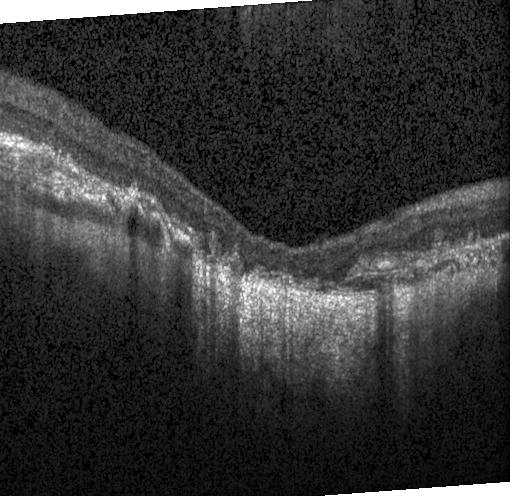 OCT line scan.
Assessment: CNV.